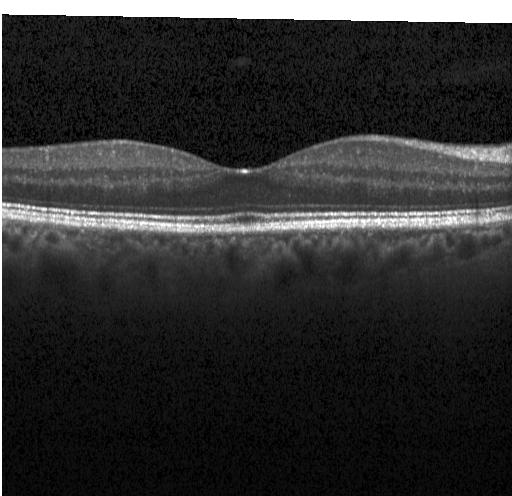
Optical coherence tomography scan
Finding: neither choroidal neovascularization, diabetic macular edema, nor drusen.